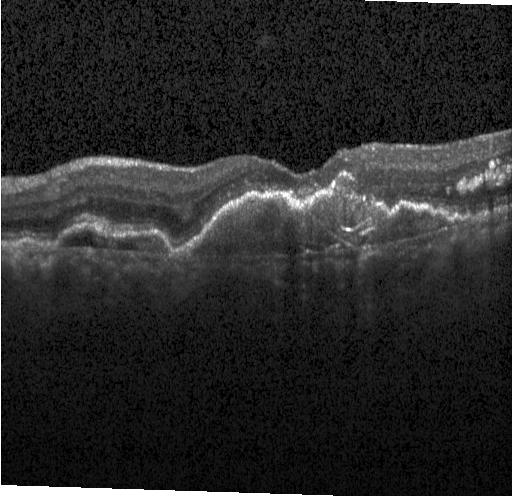

Finding: choroidal neovascularization (CNV).